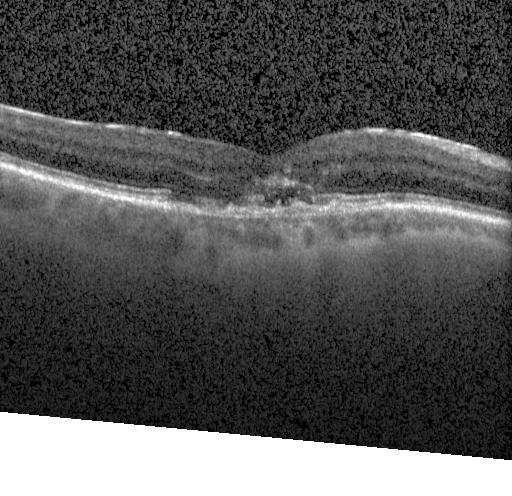 Centered on the fovea; retinal OCT B-scan — Diagnosis: a choroidal neovascular membrane.